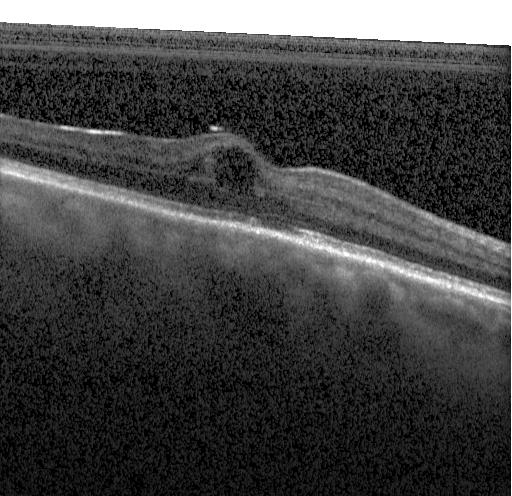 Finding: DME.